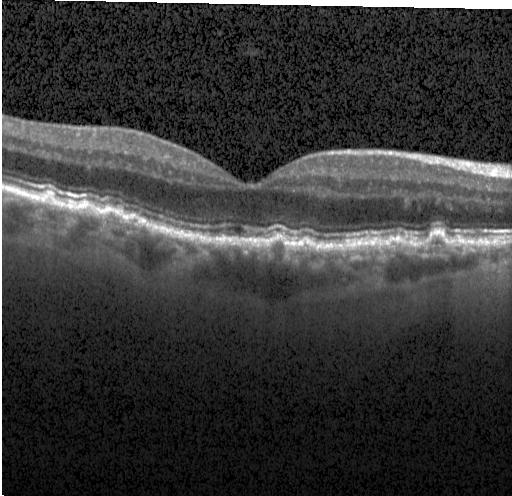

Retinal OCT B-scan; centered on the fovea. Assessment: drusen.